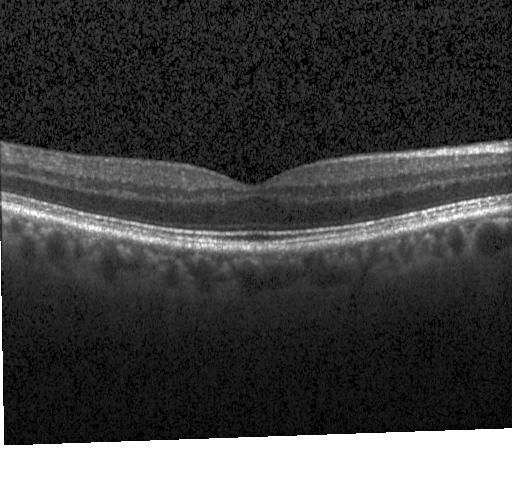 Retinal OCT B-scan · through the macula. No choroidal neovascularization, diabetic macular edema, or drusen.